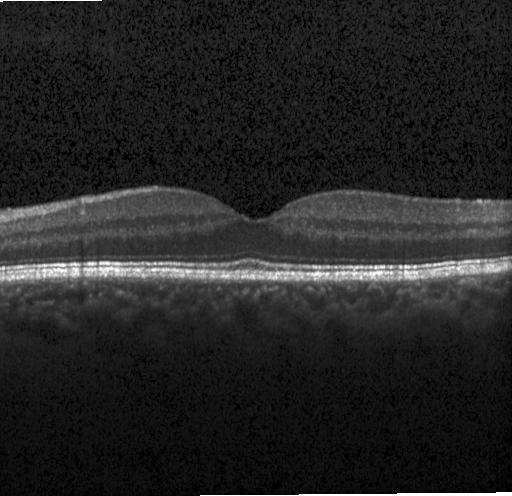 Macular OCT: no CNV, DME, or drusen.